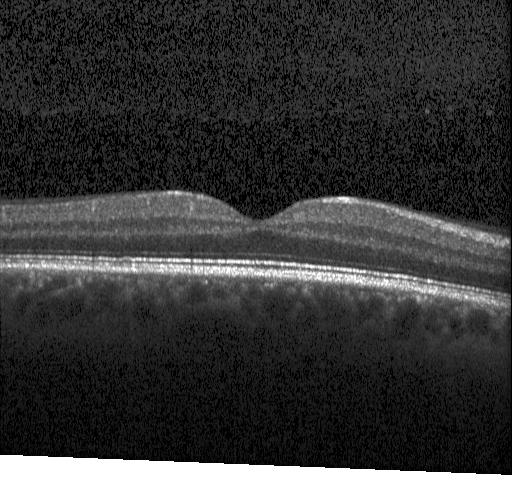
Heidelberg Spectralis · OCT B-scan · macular scan · spectral-domain optical coherence tomography — Impression: no evidence of CNV, DME, or drusen.